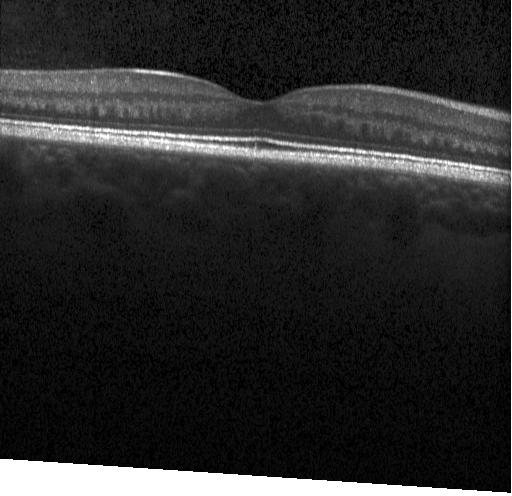
OCT line scan.
Dx: no choroidal neovascularization, no diabetic macular edema, and no drusen.